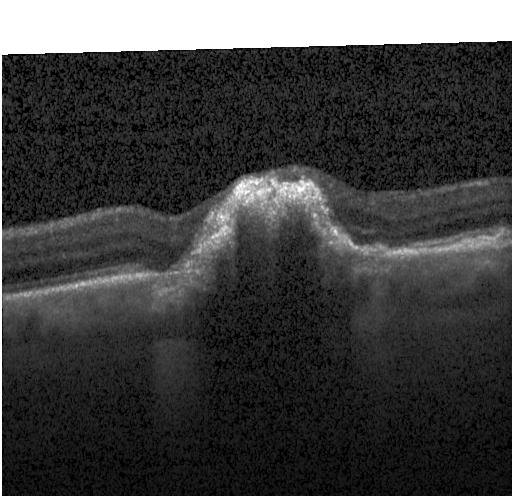 Acquired on a Heidelberg Spectralis · retinal OCT B-scan — A choroidal neovascular membrane.